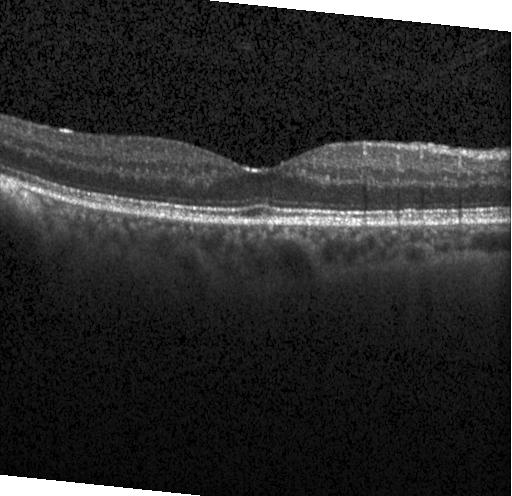

Optical coherence tomography B-scan. Macular scan. Heidelberg Spectralis OCT system. Spectral-domain OCT
Impression: no evidence of CNV, DME, or drusen.